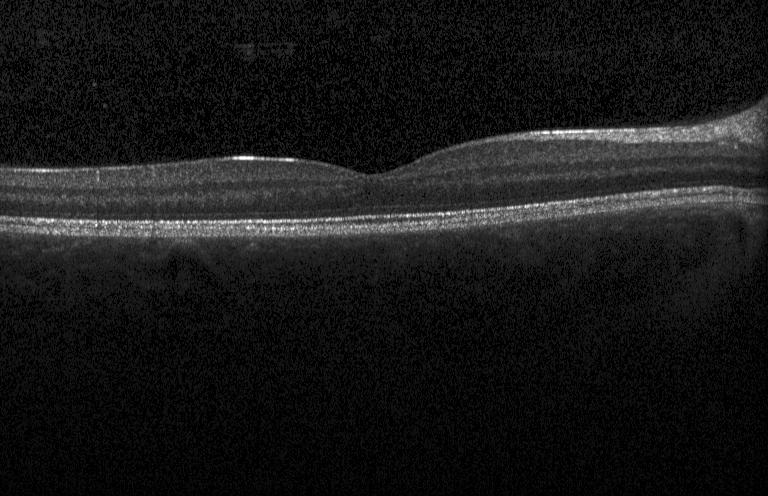 OCT B-scan
The scan shows neither choroidal neovascularization, diabetic macular edema, nor drusen.